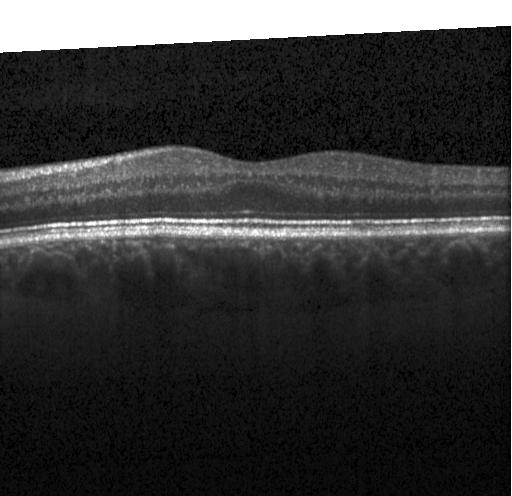
Centered on the fovea; OCT line scan. Impression: no evidence of choroidal neovascularization, diabetic macular edema, or drusen.